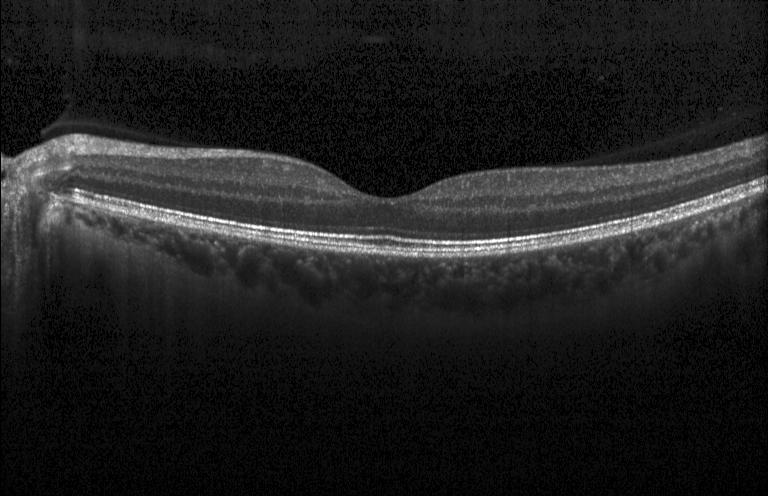 Spectral-domain optical coherence tomography, optical coherence tomography B-scan, centered on the fovea. OCT finding: no choroidal neovascularization, diabetic macular edema, or drusen.